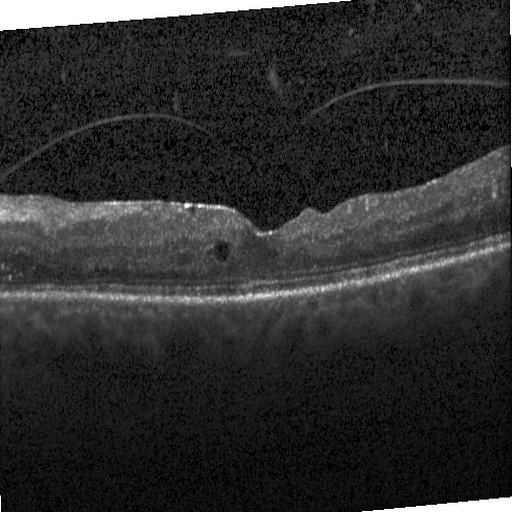 Centered on the fovea, optical coherence tomography B-scan, SD-OCT, instrument: Heidelberg Spectralis — Impression: diabetic macular edema (DME).